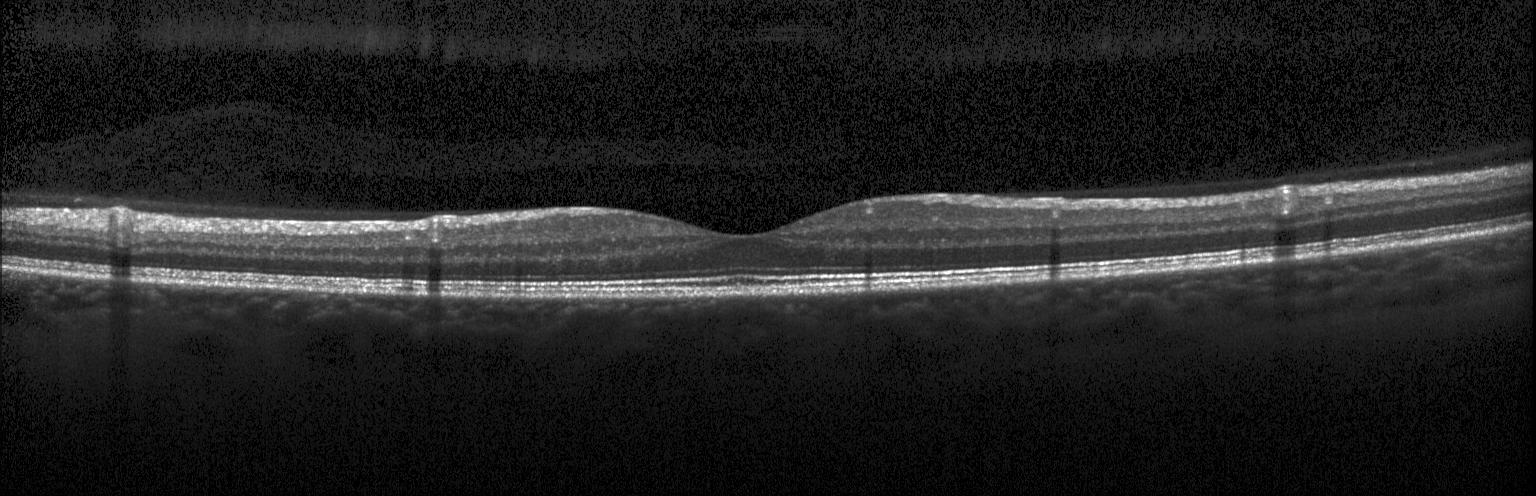 Centered on the fovea; retinal OCT B-scan; spectral-domain OCT; Heidelberg Spectralis OCT system.
Dx: no choroidal neovascularization, no diabetic macular edema, and no drusen.